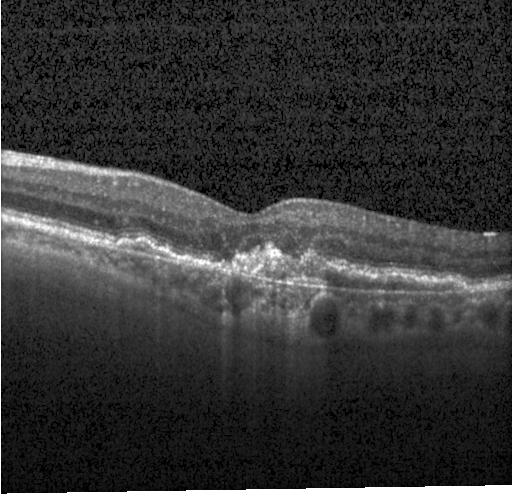
Diagnosis: choroidal neovascularization (CNV).